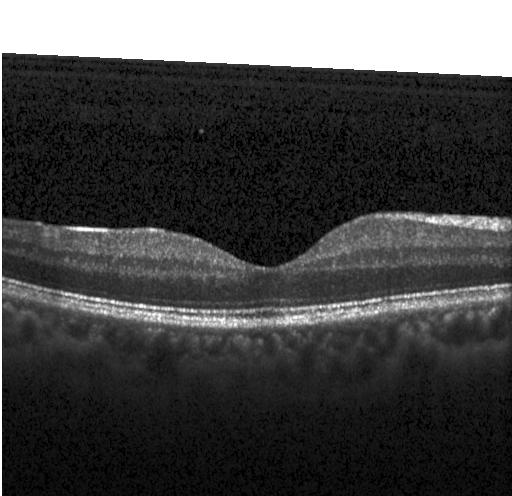
Diagnosis: no CNV, no DME, and no drusen.